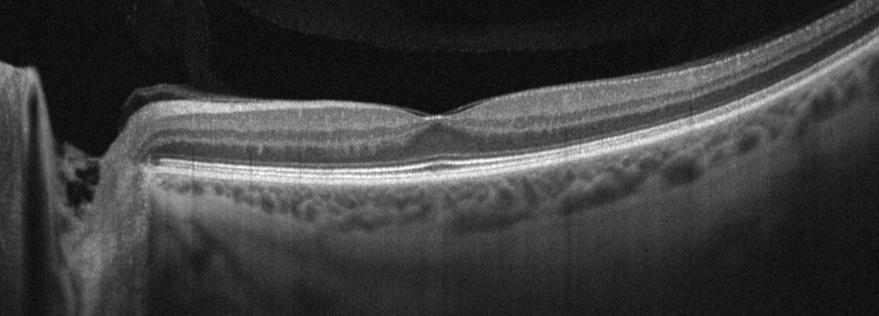 Acquired on an Optovue Avanti RTVue XR; optical coherence tomography scan. Dx: no evidence of AMD, DME, ERM, RAO, RVO, or VID.